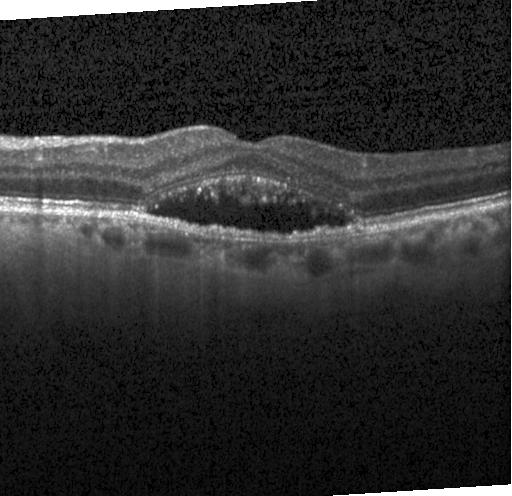 Optical coherence tomography B-scan — Assessment: choroidal neovascularization.